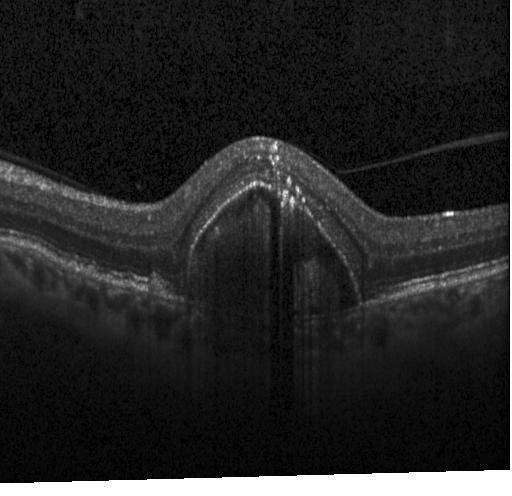 Macular OCT demonstrating a choroidal neovascular membrane.